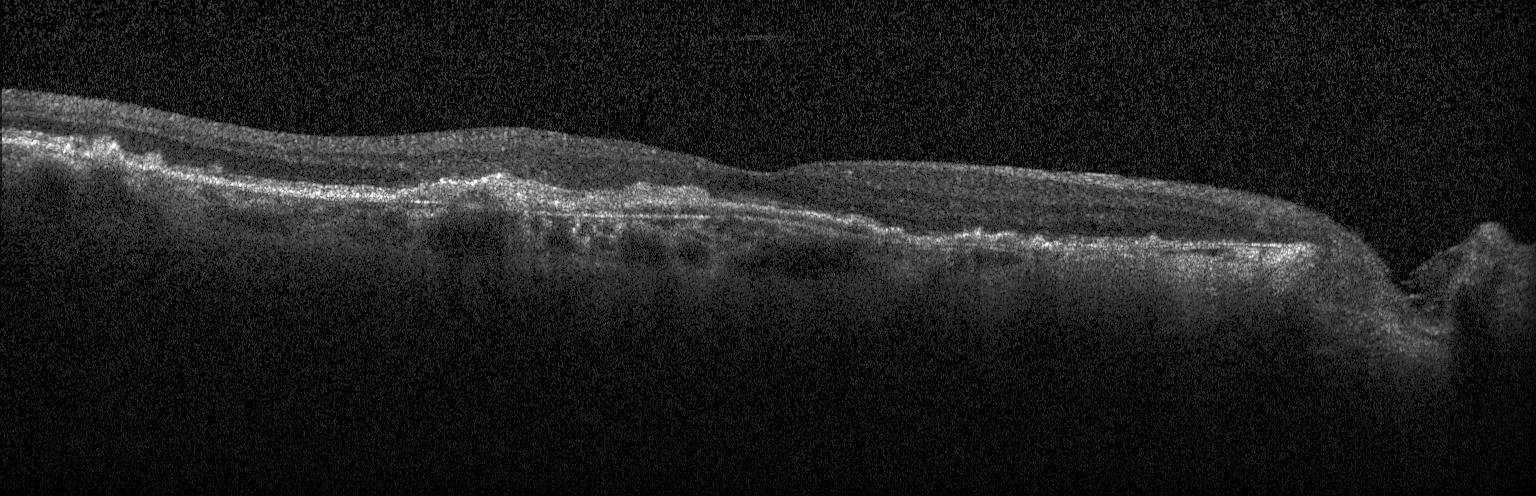
Through the macula; spectral-domain optical coherence tomography; acquired on a Heidelberg Spectralis; optical coherence tomography B-scan — Diagnosis: choroidal neovascularization.